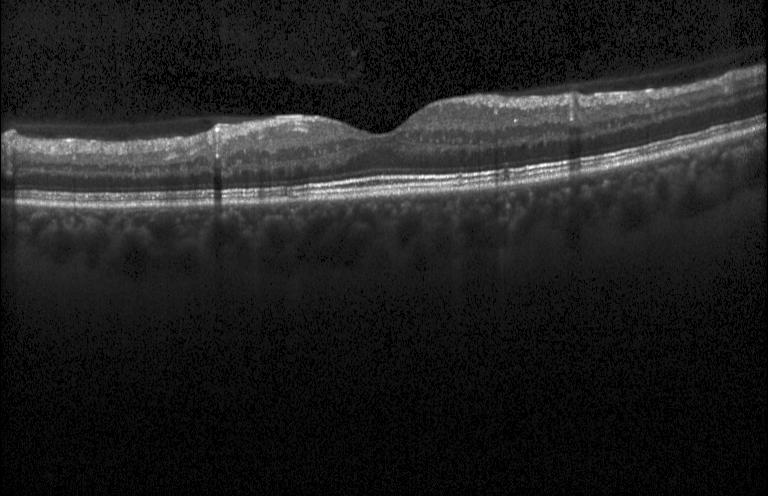
The scan shows no choroidal neovascularization, no diabetic macular edema, and no drusen.